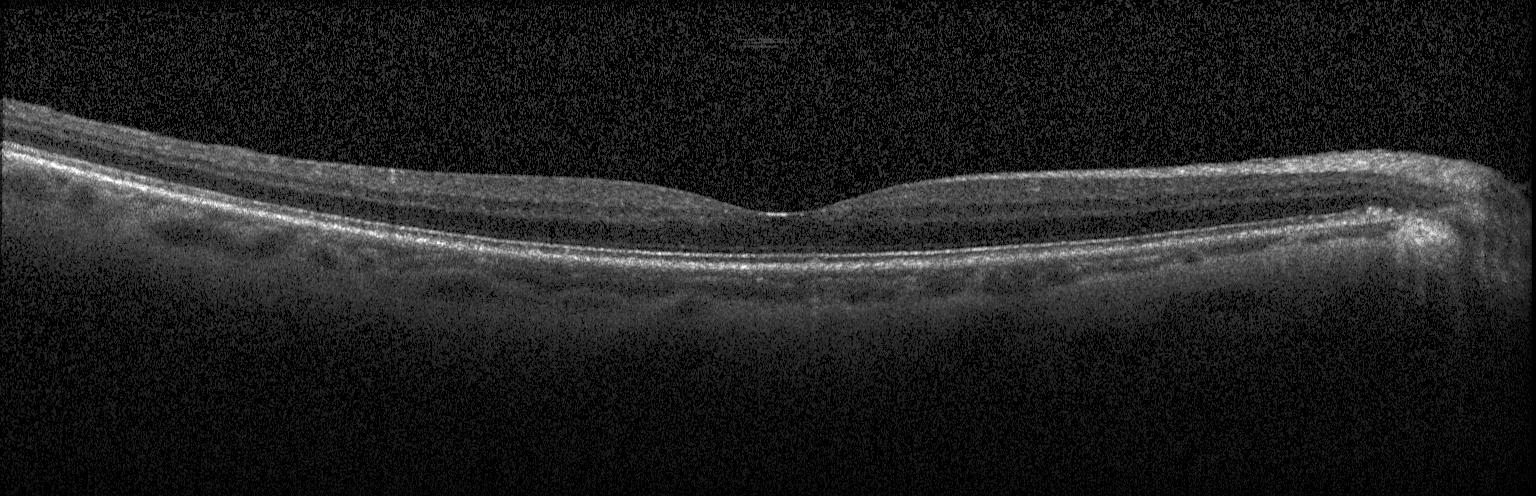 The scan shows neither choroidal neovascularization, diabetic macular edema, nor drusen.